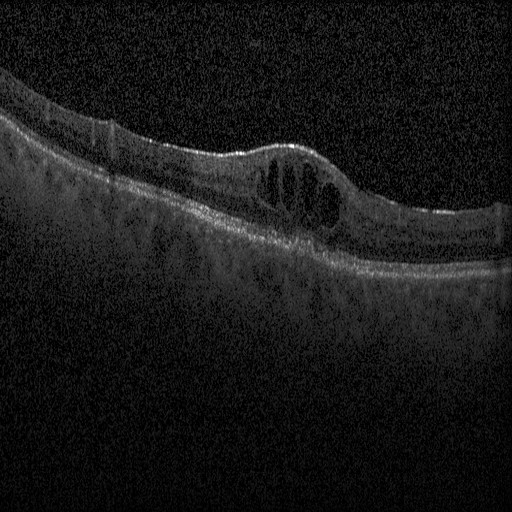 Macular OCT demonstrating diabetic macular edema.